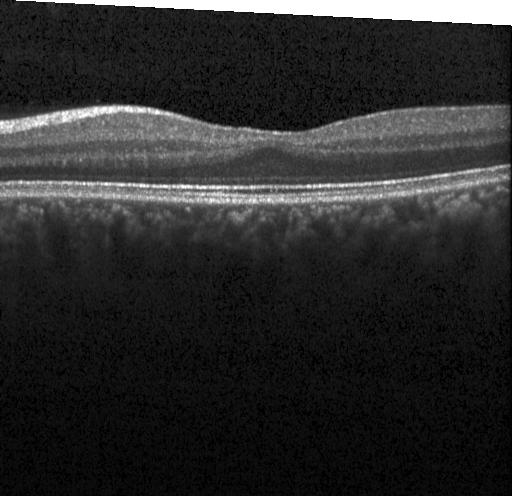
OCT line scan. This B-scan demonstrates no choroidal neovascularization, diabetic macular edema, or drusen.